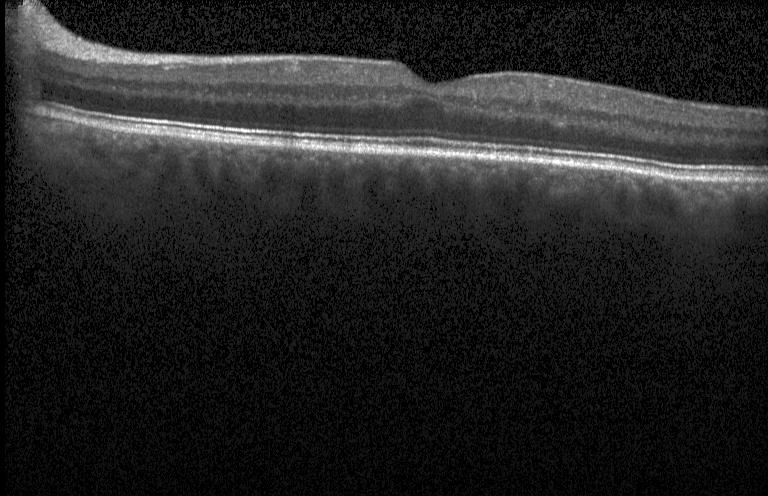
Optical coherence tomography scan. The scan shows no evidence of choroidal neovascularization, diabetic macular edema, or drusen.